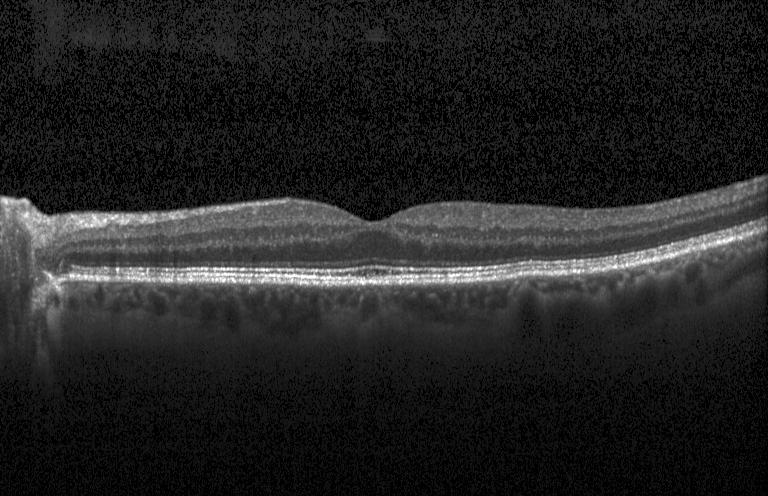

OCT B-scan showing no CNV, DME, or drusen.